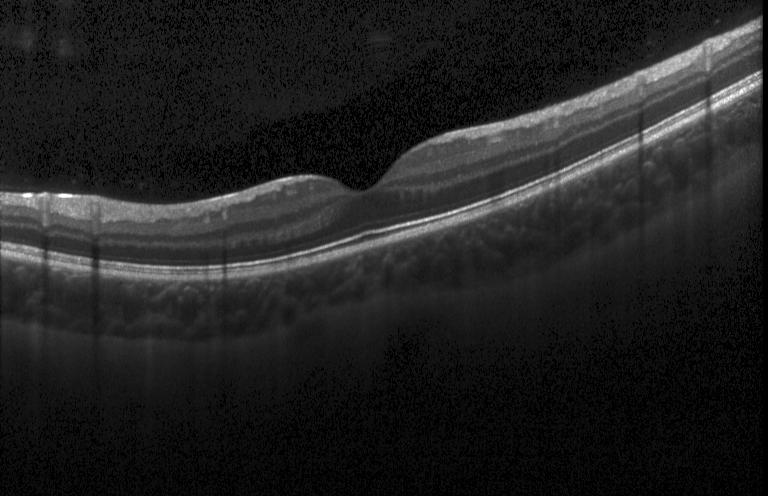 Fovea-centered. Spectral-domain OCT. Optical coherence tomography scan. Instrument: Heidelberg Spectralis.
Impression: no evidence of choroidal neovascularization, diabetic macular edema, or drusen.